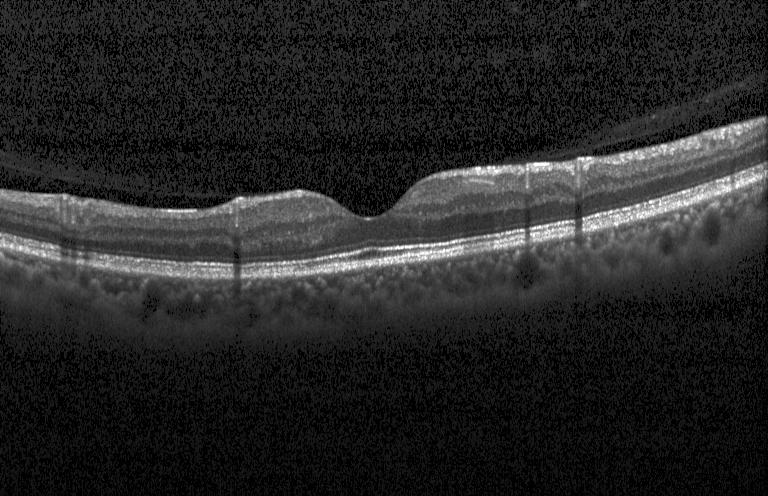
Diagnosis: neither CNV, DME, nor drusen.